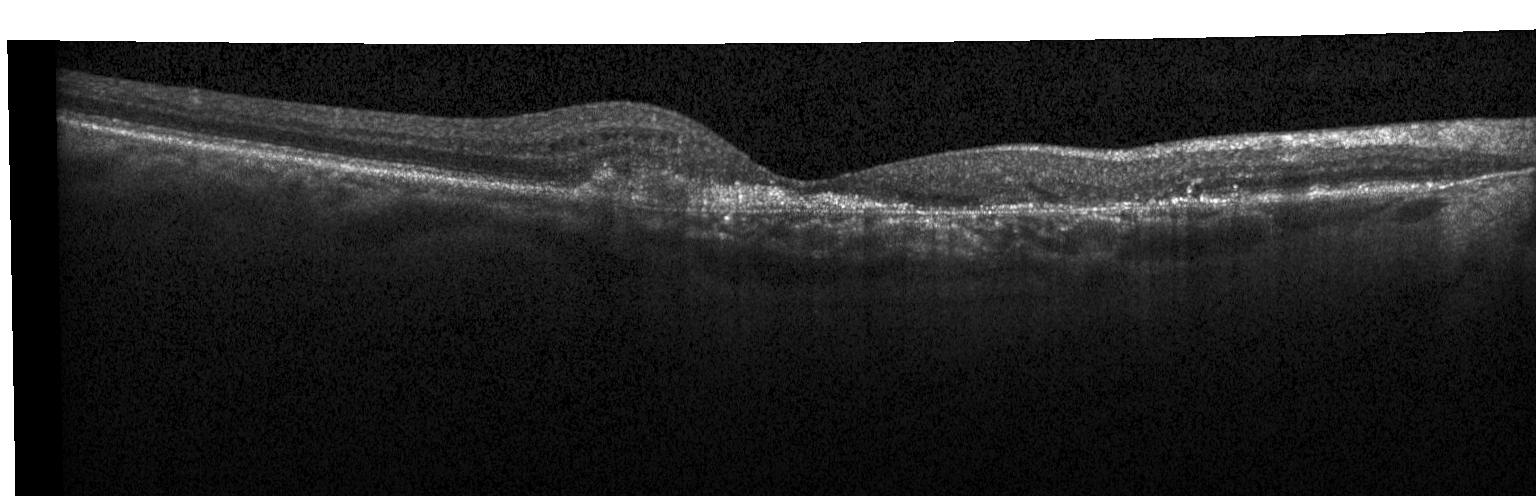 Optical coherence tomography scan — The scan shows a choroidal neovascular membrane.